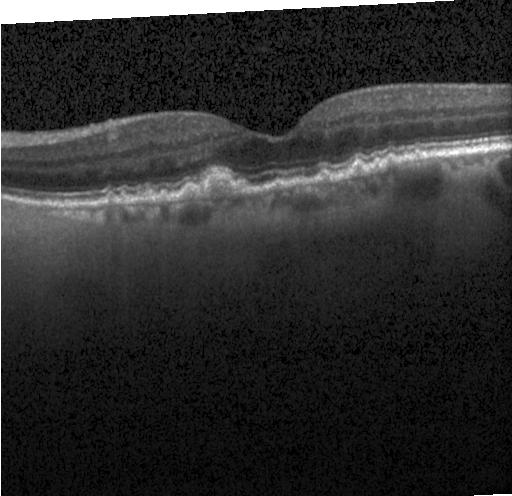

Optical coherence tomography scan — Finding: multiple drusen.